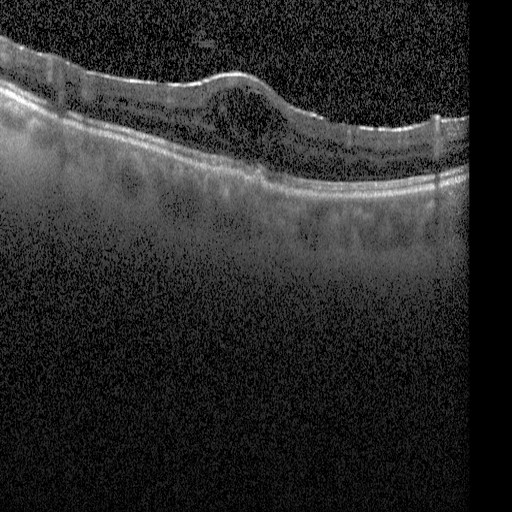 Impression: DME.